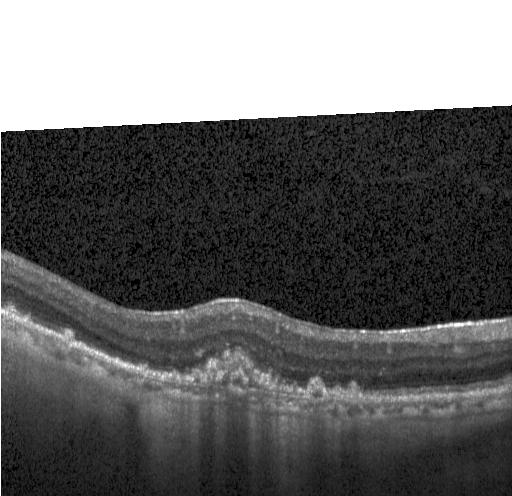 Centered on the fovea; SD-OCT; Heidelberg Spectralis OCT system; OCT line scan — Assessment: choroidal neovascularization (CNV).